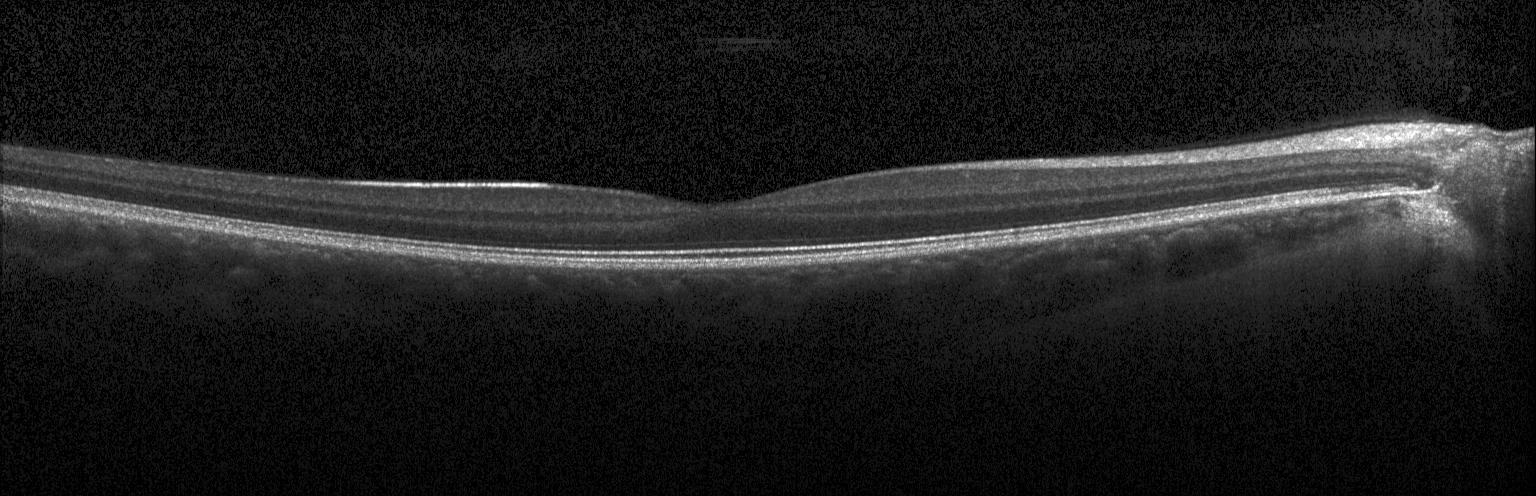
Macular OCT demonstrating no evidence of choroidal neovascularization, diabetic macular edema, or drusen.